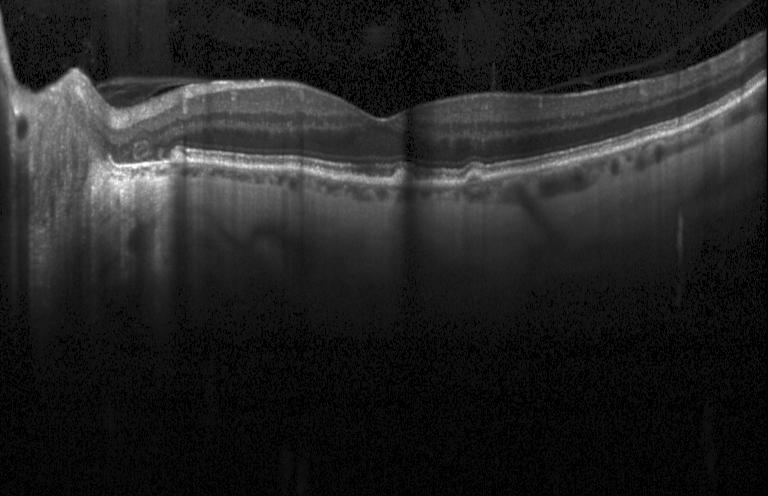 Heidelberg Spectralis OCT system; retinal OCT cross-section — Impression: multiple drusen.